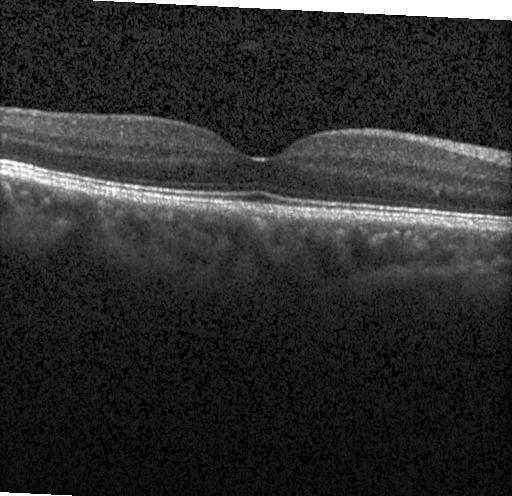

Acquired on a Heidelberg Spectralis · OCT line scan · SD-OCT · horizontal scan through the fovea.
Impression: no choroidal neovascularization, diabetic macular edema, or drusen.